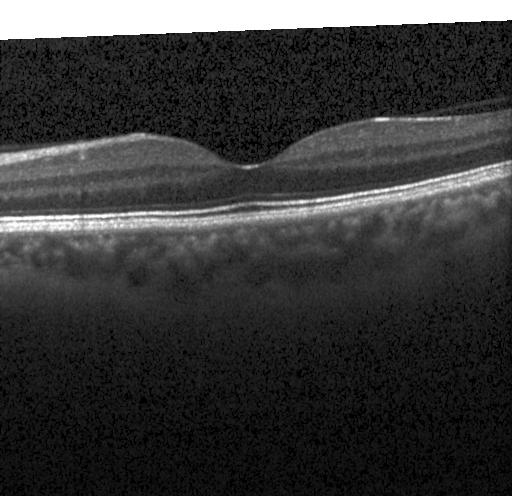
Diagnosis: no evidence of choroidal neovascularization, diabetic macular edema, or drusen.